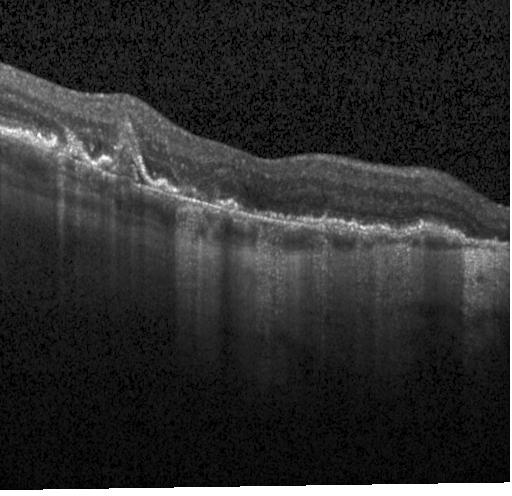

Spectral-domain OCT B-scan: a choroidal neovascular membrane.